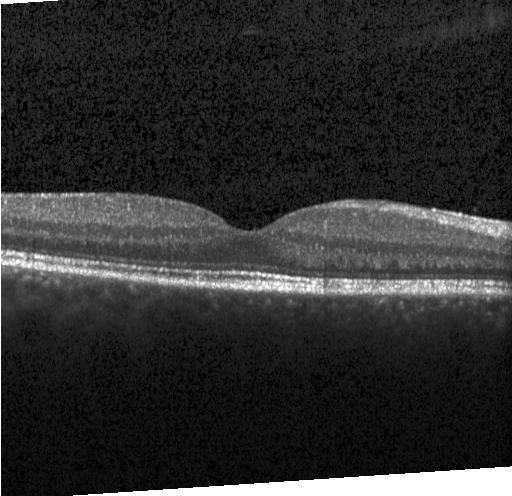 OCT scan showing no evidence of choroidal neovascularization, diabetic macular edema, or drusen.